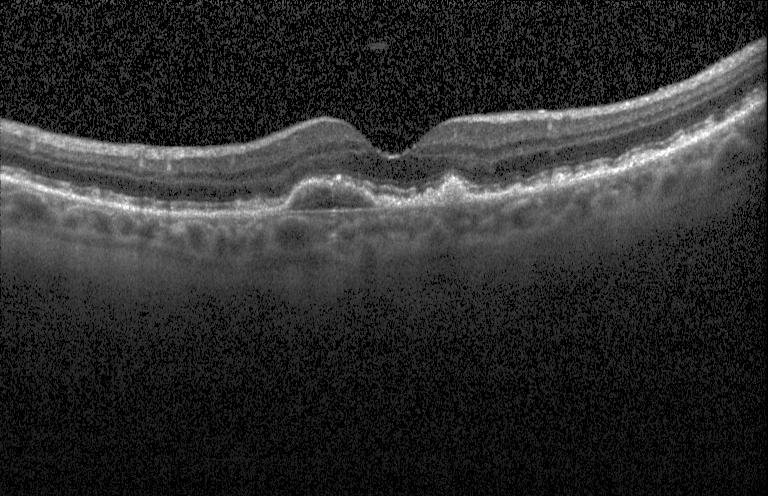
OCT line scan. Diagnosis: choroidal neovascularization.